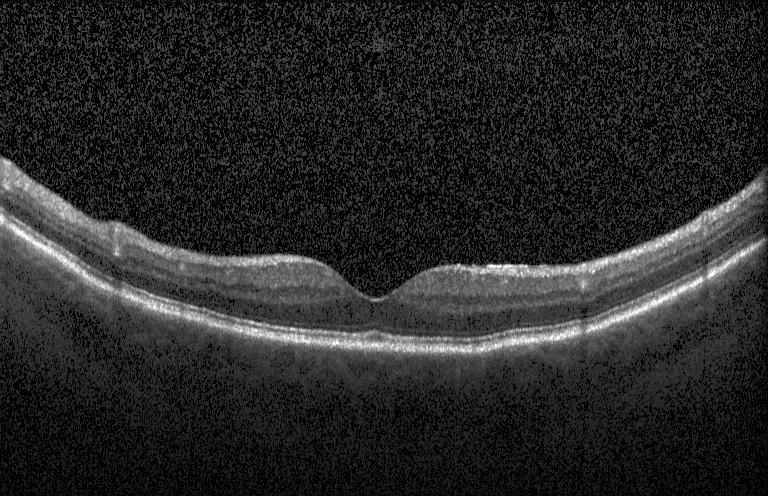

OCT B-scan. Spectral-domain OCT. Diagnosis: no CNV, DME, or drusen.